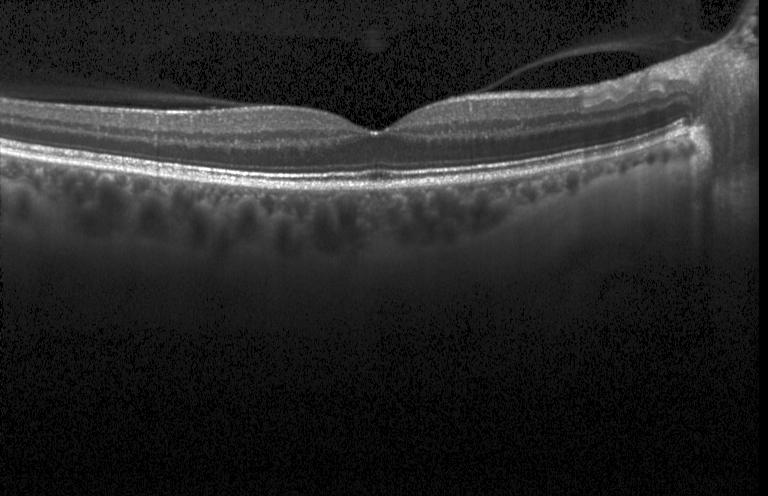

Assessment: no CNV, no DME, and no drusen.